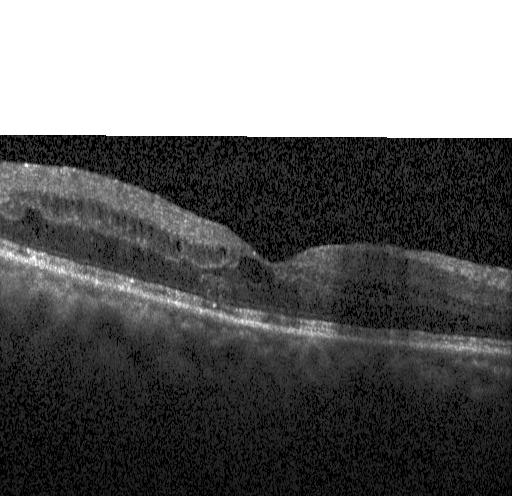

Spectral-domain OCT; retinal OCT cross-section; instrument: Heidelberg Spectralis; horizontal scan through the fovea
Finding: DME.